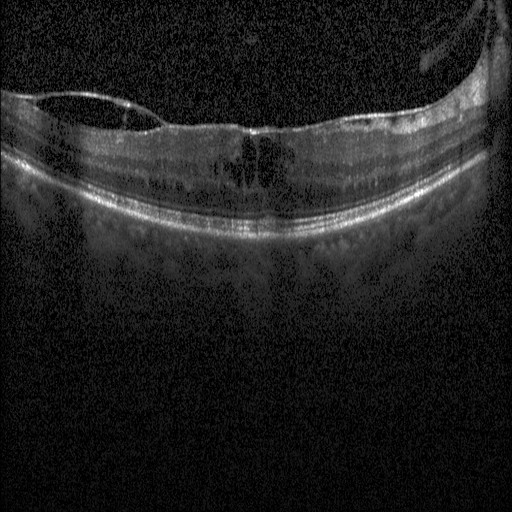 Heidelberg Spectralis, retinal OCT cross-section, SD-OCT, fovea-centered. Finding: diabetic macular edema (DME).